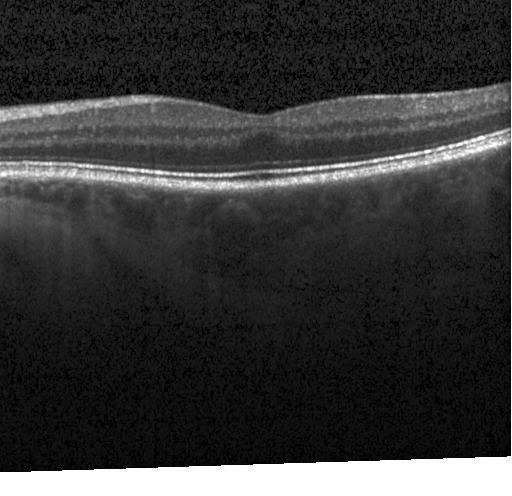

Macular OCT: neither choroidal neovascularization, diabetic macular edema, nor drusen.